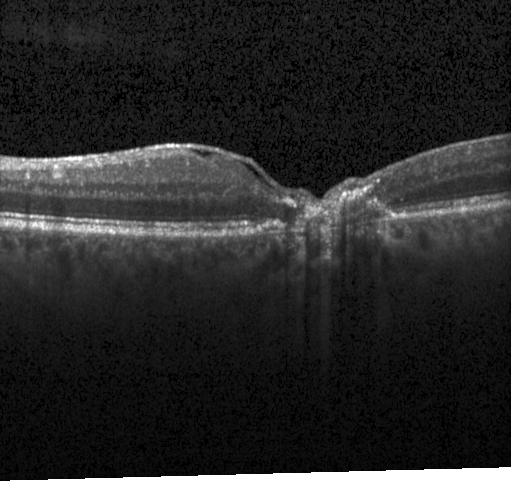
Spectral-domain OCT, optical coherence tomography B-scan, instrument: Heidelberg Spectralis, horizontal scan through the fovea. The scan shows a choroidal neovascular membrane.